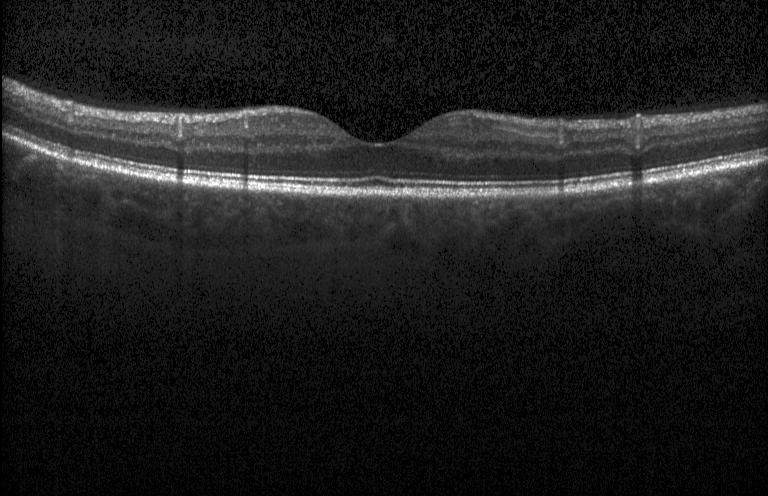 Spectral-domain OCT, OCT B-scan, macular scan — Impression: no evidence of choroidal neovascularization, diabetic macular edema, or drusen.